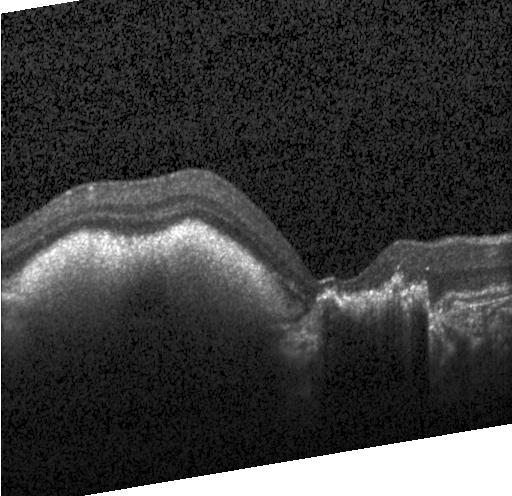 This B-scan demonstrates a choroidal neovascular membrane.